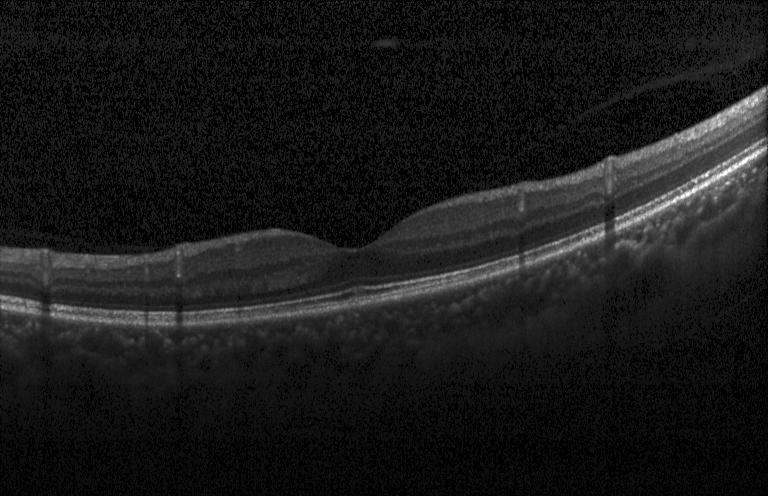

OCT finding: neither choroidal neovascularization, diabetic macular edema, nor drusen.